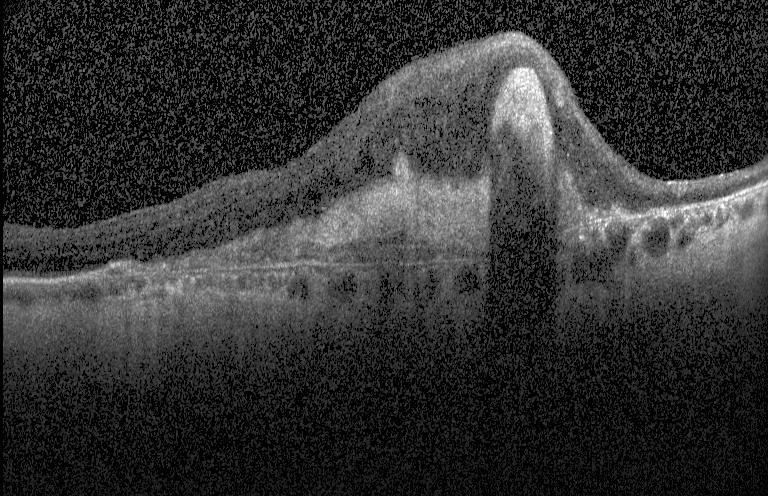
OCT line scan — A choroidal neovascular membrane.